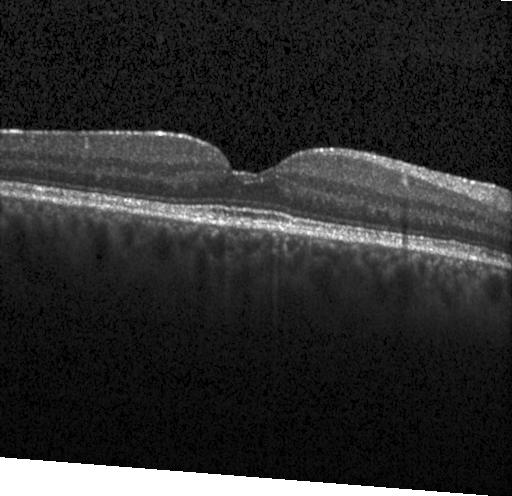
Diagnosis: no evidence of CNV, DME, or drusen.